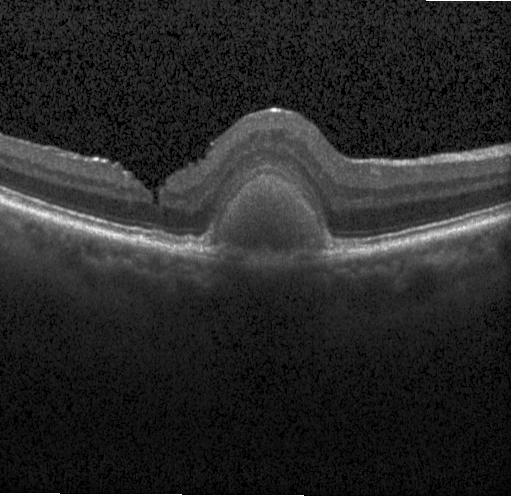
OCT finding: a choroidal neovascular membrane.